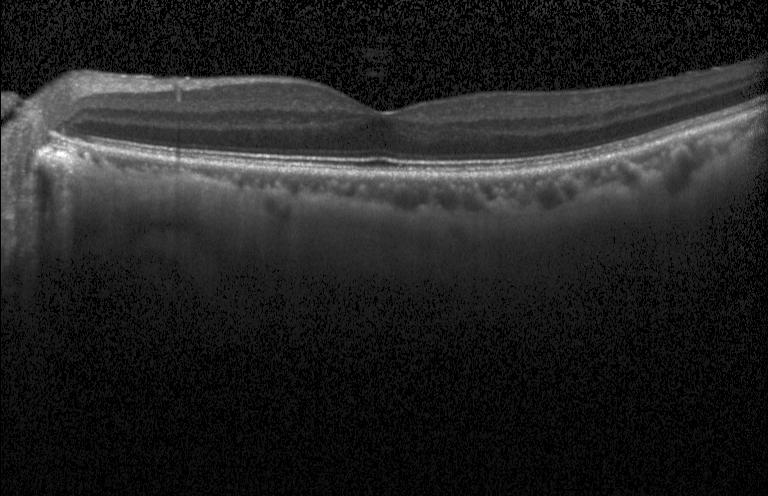 Impression: no evidence of choroidal neovascularization, diabetic macular edema, or drusen.